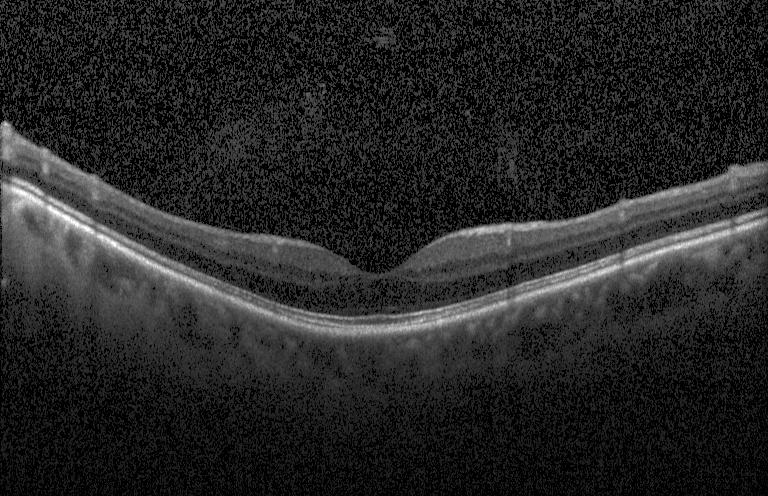

Spectral-domain OCT; horizontal scan through the fovea; Heidelberg Spectralis OCT system; OCT line scan.
Assessment: neither choroidal neovascularization, diabetic macular edema, nor drusen.